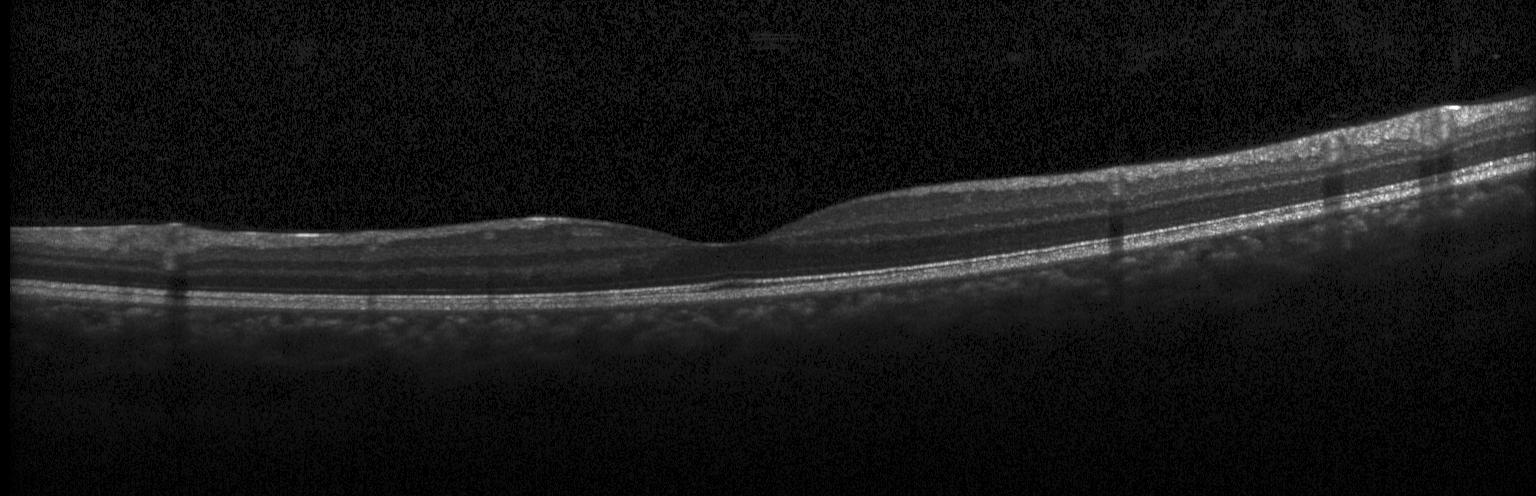
Centered on the fovea, Heidelberg Spectralis, retinal OCT cross-section, spectral-domain optical coherence tomography. This B-scan demonstrates no CNV, DME, or drusen.